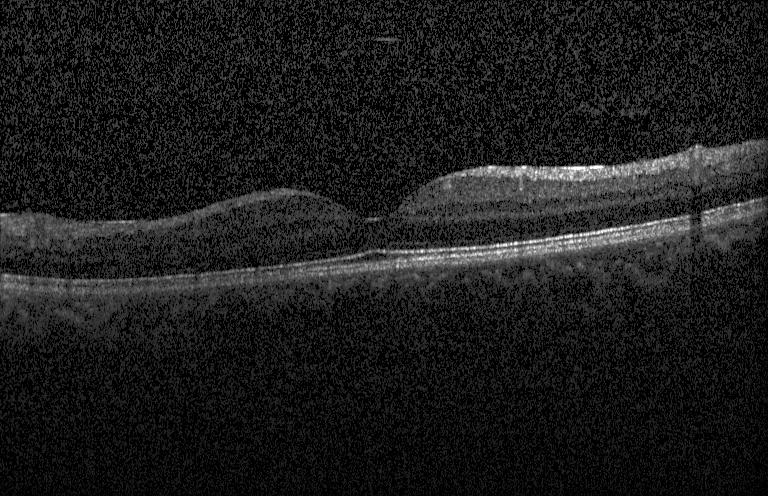

Acquired on a Heidelberg Spectralis · OCT B-scan
Dx: no choroidal neovascularization, diabetic macular edema, or drusen.